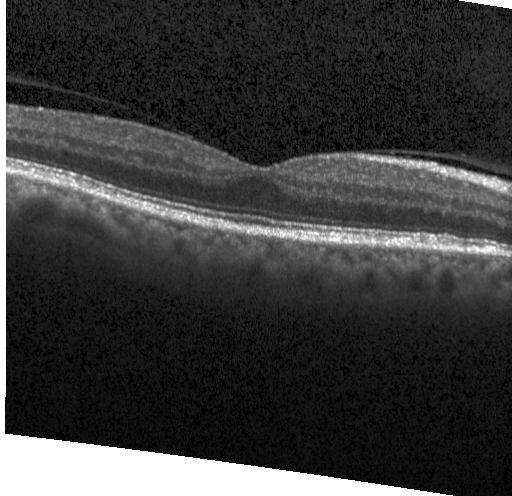

Macular OCT: no choroidal neovascularization, diabetic macular edema, or drusen.